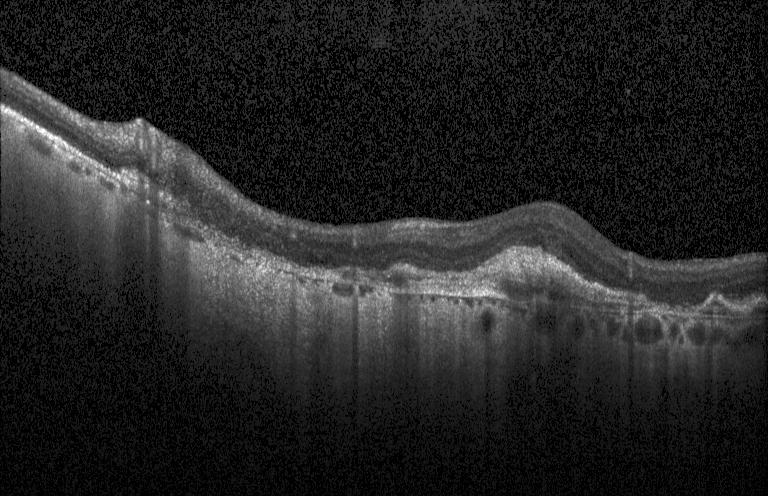

Spectral-domain OCT. Horizontal scan through the fovea. Optical coherence tomography B-scan. Diagnosis: choroidal neovascularization.